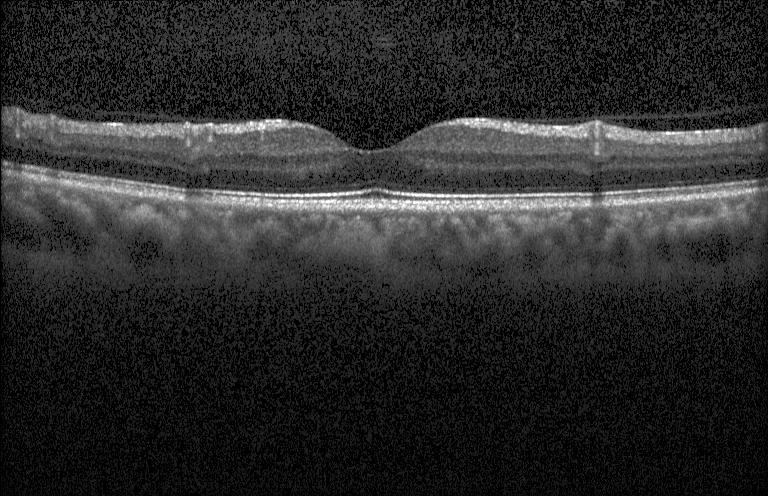

Acquired on a Heidelberg Spectralis. Horizontal scan through the fovea. SD-OCT. OCT B-scan.
Diagnosis: no choroidal neovascularization, diabetic macular edema, or drusen.